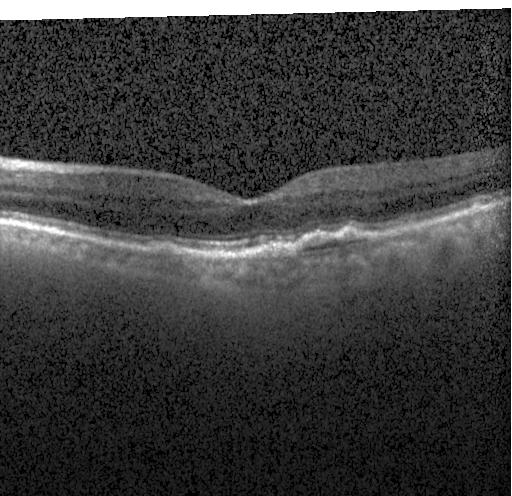 Acquired on a Heidelberg Spectralis · retinal OCT B-scan
Diagnosis: choroidal neovascularization (CNV).